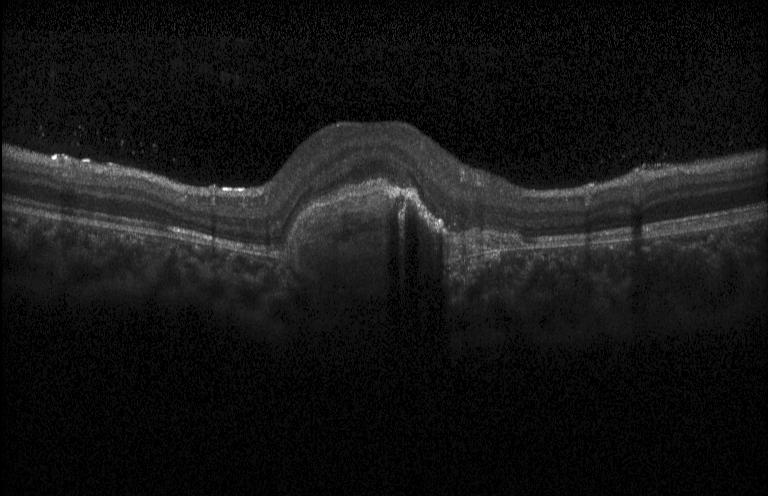
SD-OCT; optical coherence tomography scan.
Impression: a choroidal neovascular membrane.